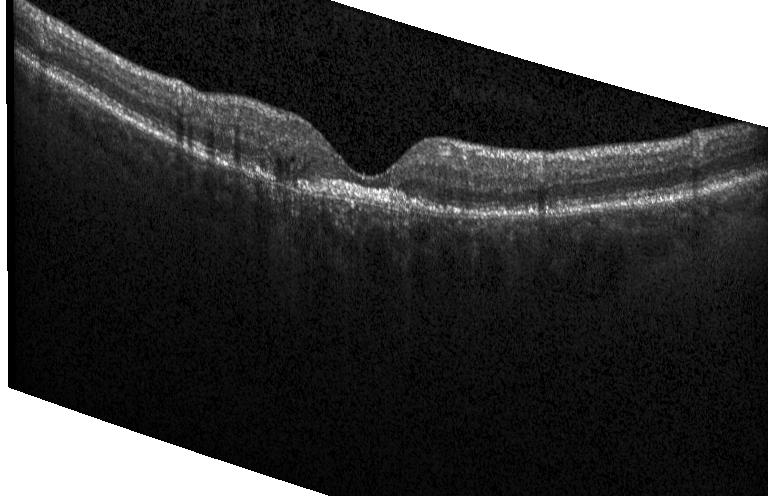

Retinal OCT cross-section showing choroidal neovascularization (CNV).